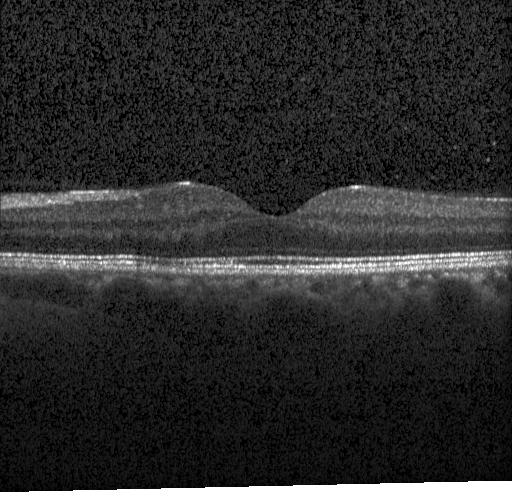

Optical coherence tomography B-scan · spectral-domain OCT · Heidelberg Spectralis OCT system. Diagnosis: no choroidal neovascularization, no diabetic macular edema, and no drusen.